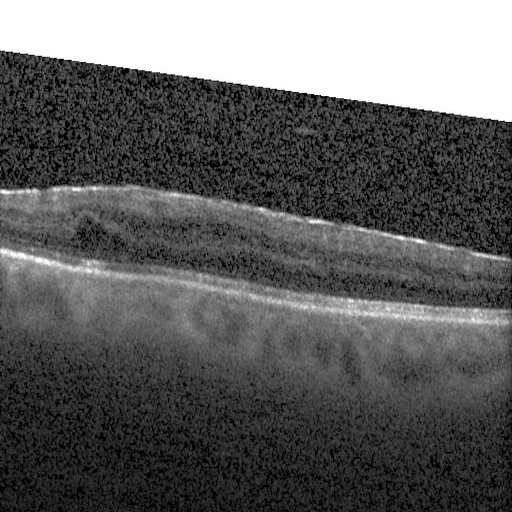 Acquired on a Heidelberg Spectralis, OCT B-scan, spectral-domain OCT. Impression: DME.